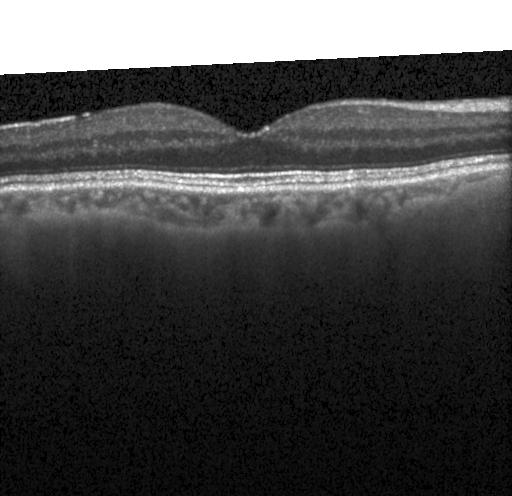

OCT finding: no evidence of choroidal neovascularization, diabetic macular edema, or drusen.